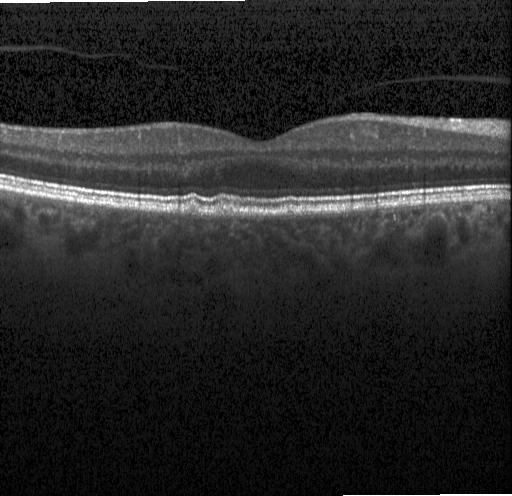

Optical coherence tomography B-scan
Impression: sub-RPE drusenoid deposits.